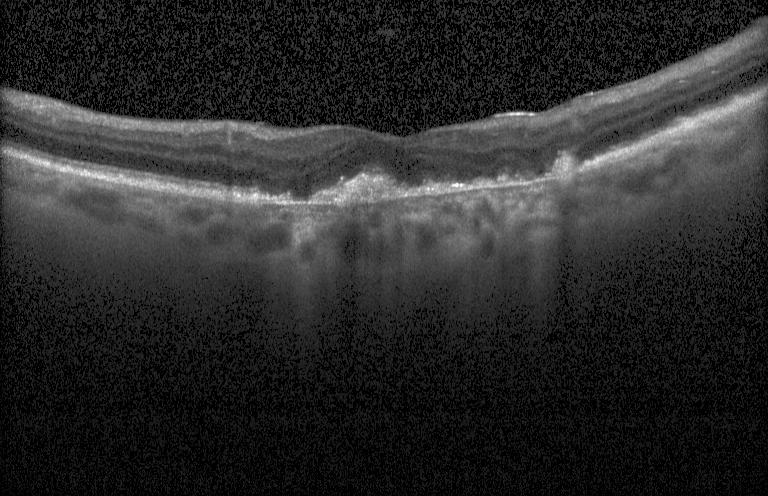 Impression: a choroidal neovascular membrane.